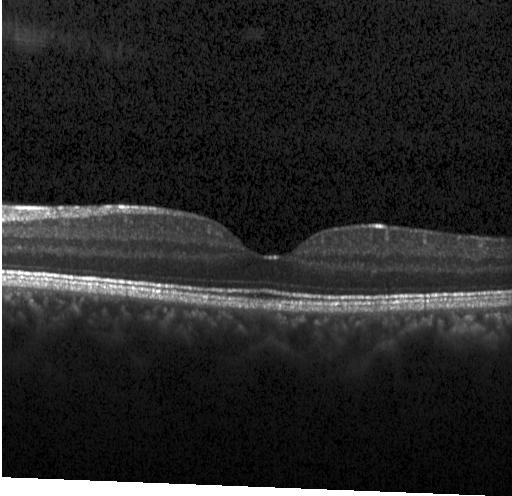 Retinal OCT cross-section showing no CNV, DME, or drusen.